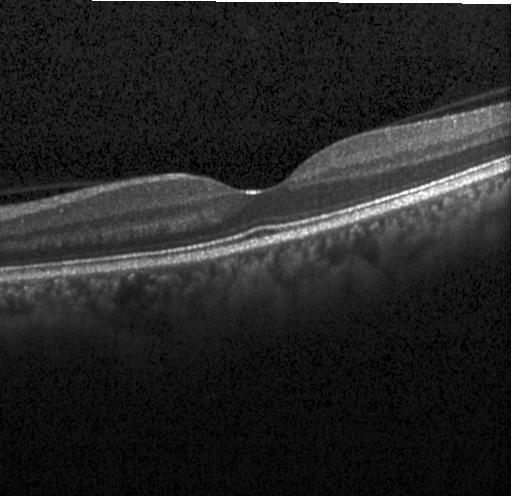 Acquired on a Heidelberg Spectralis; SD-OCT; OCT line scan; centered on the fovea — Assessment: no choroidal neovascularization, no diabetic macular edema, and no drusen.